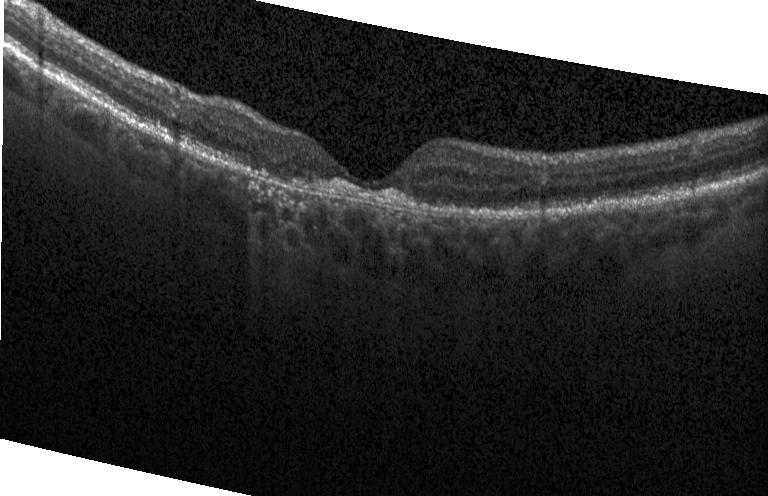
Acquired on a Heidelberg Spectralis · OCT B-scan.
Impression: choroidal neovascularization.